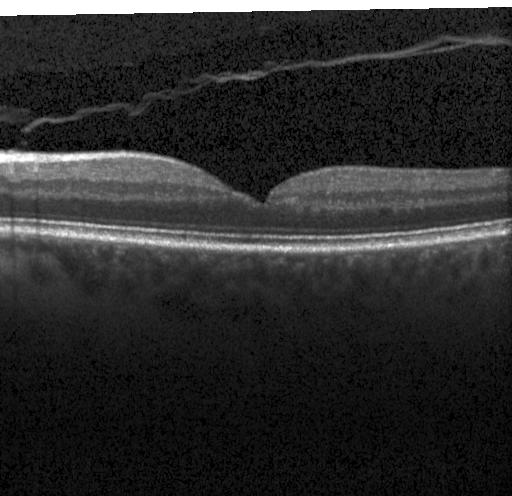 Optical coherence tomography scan
Finding: no choroidal neovascularization, diabetic macular edema, or drusen.